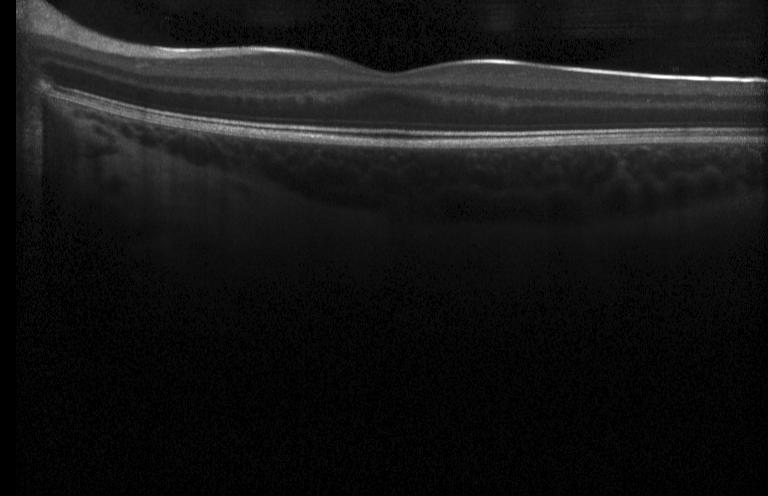
Optical coherence tomography scan; acquired on a Heidelberg Spectralis
The scan shows no choroidal neovascularization, diabetic macular edema, or drusen.